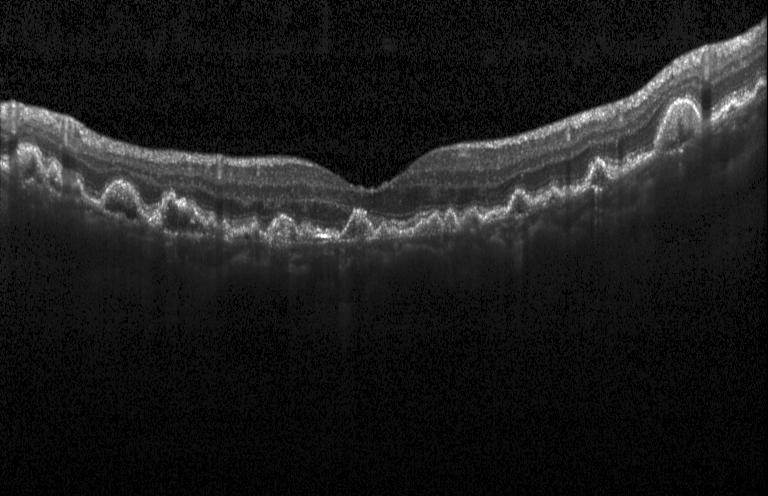
OCT B-scan. Assessment: a choroidal neovascular membrane.